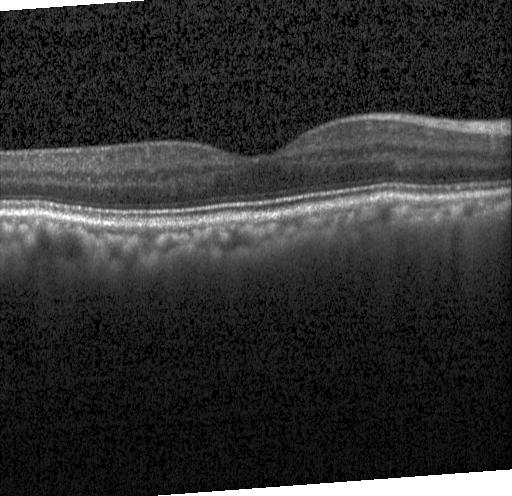 Optical coherence tomography scan
No choroidal neovascularization, no diabetic macular edema, and no drusen.